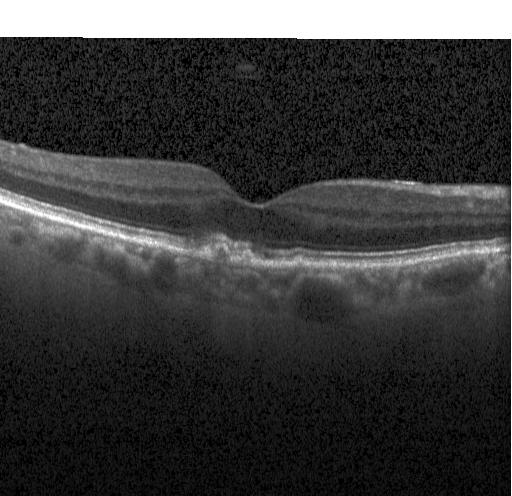
OCT line scan
Finding: sub-RPE drusenoid deposits.